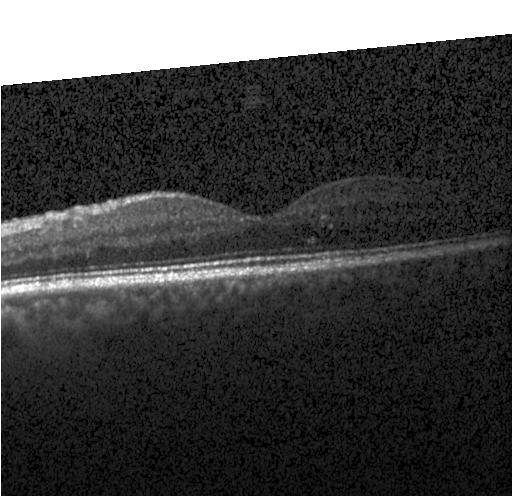

This B-scan demonstrates neither choroidal neovascularization, diabetic macular edema, nor drusen.